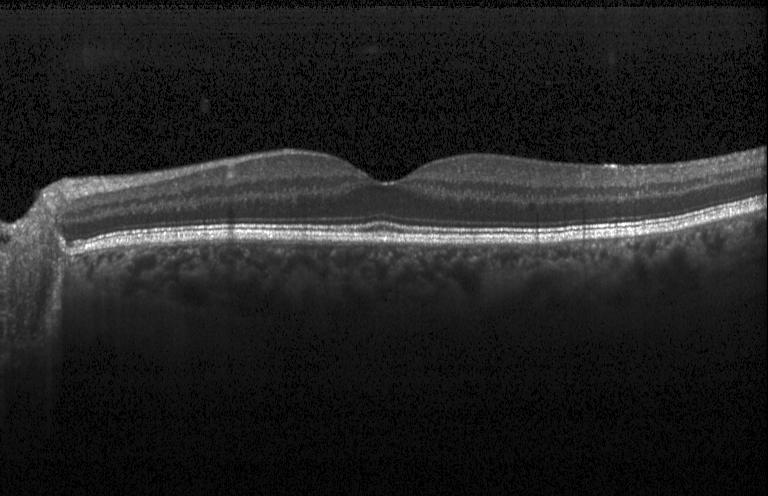 Optical coherence tomography B-scan, Heidelberg Spectralis OCT system.
Finding: neither choroidal neovascularization, diabetic macular edema, nor drusen.